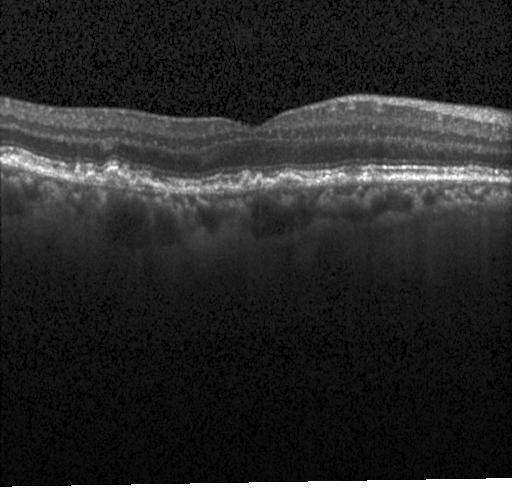

Macular OCT: drusen.